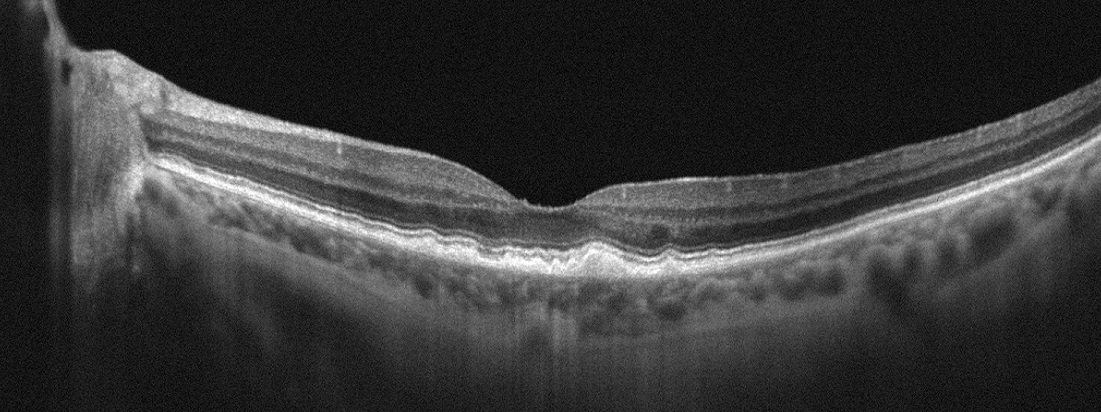 OCT finding: age-related macular degeneration.